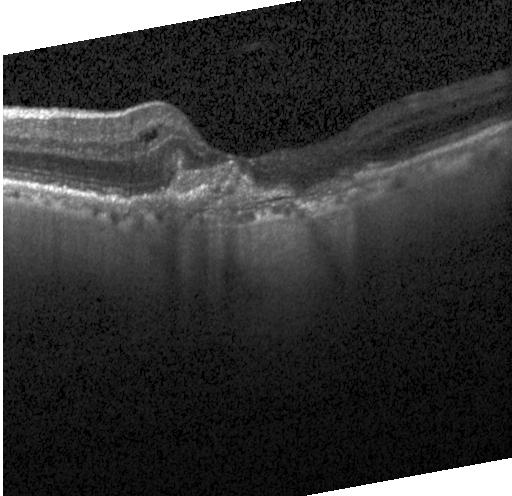
OCT line scan. Macular scan.
Assessment: a choroidal neovascular membrane.